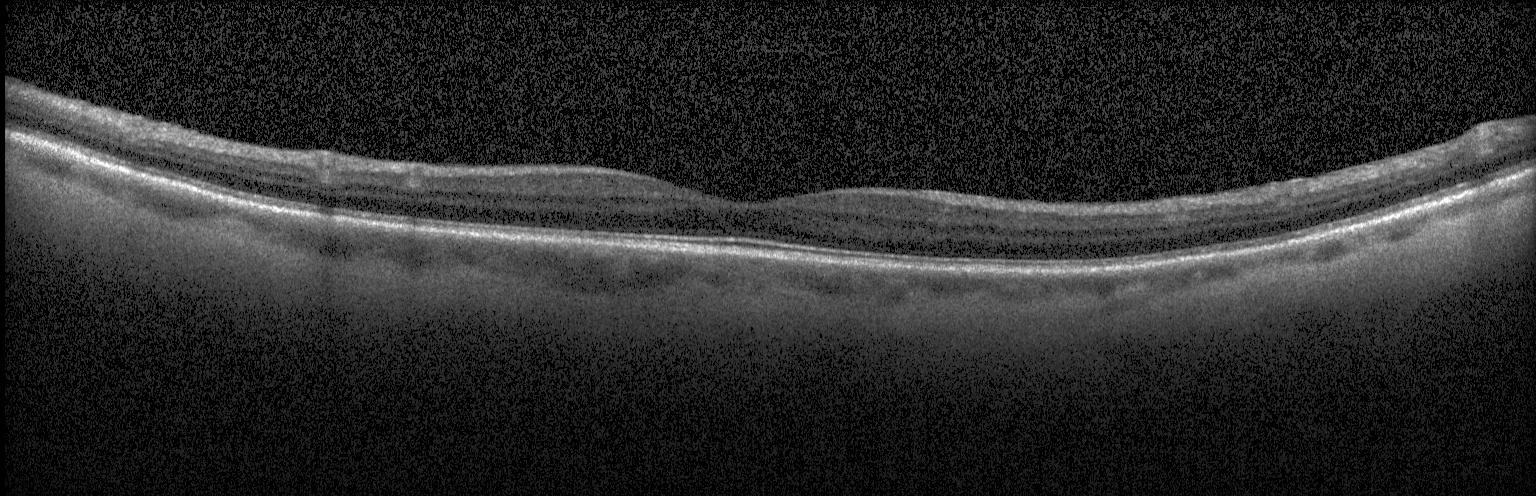
Optical coherence tomography B-scan, spectral-domain optical coherence tomography. Impression: no choroidal neovascularization, diabetic macular edema, or drusen.